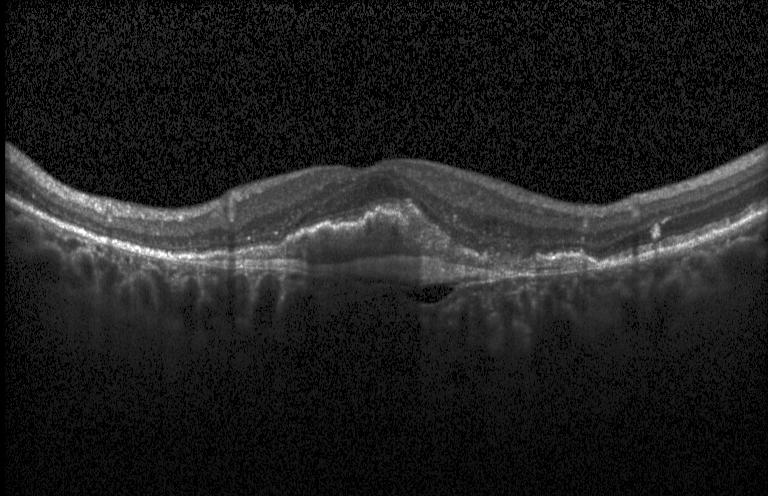 SD-OCT; optical coherence tomography B-scan.
This B-scan demonstrates choroidal neovascularization (CNV).